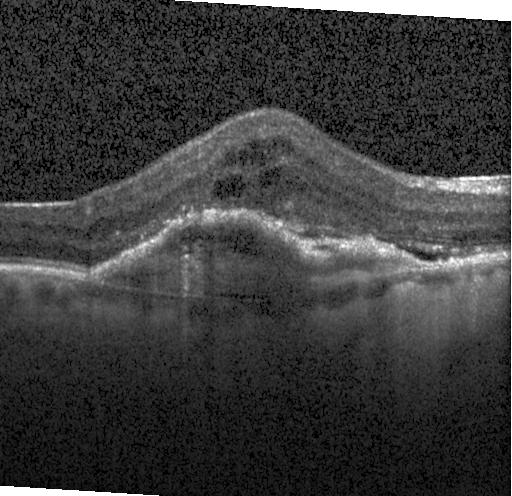

Spectral-domain OCT; instrument: Heidelberg Spectralis; OCT B-scan
Dx: a choroidal neovascular membrane.